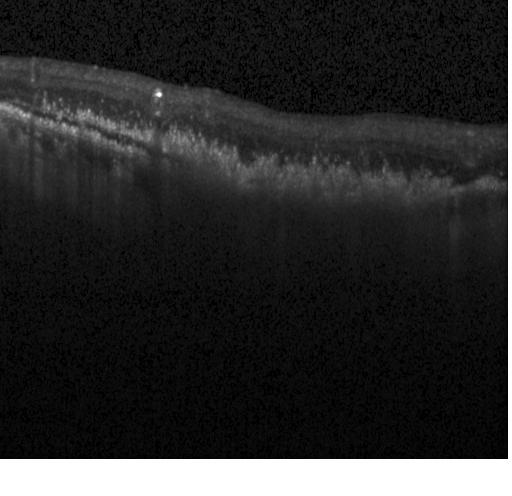 Retinal OCT B-scan.
Assessment: choroidal neovascularization.